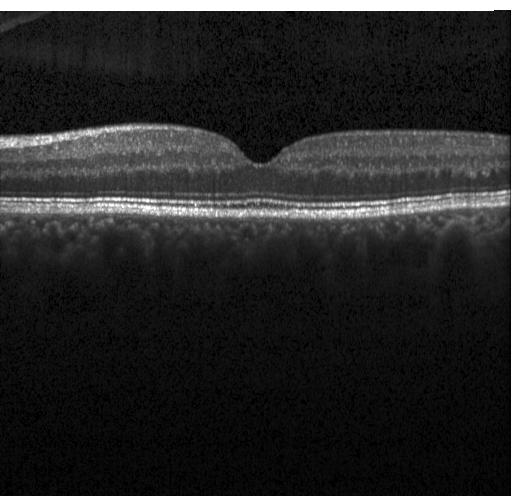

Acquired on a Heidelberg Spectralis, optical coherence tomography scan, SD-OCT, through the macula
Finding: neither choroidal neovascularization, diabetic macular edema, nor drusen.